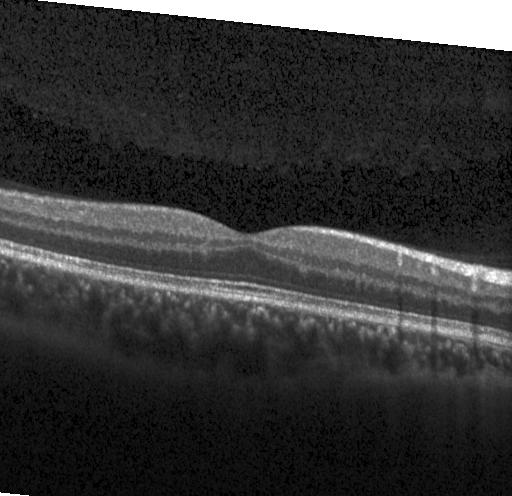 Retinal OCT B-scan. Finding: no CNV, DME, or drusen.